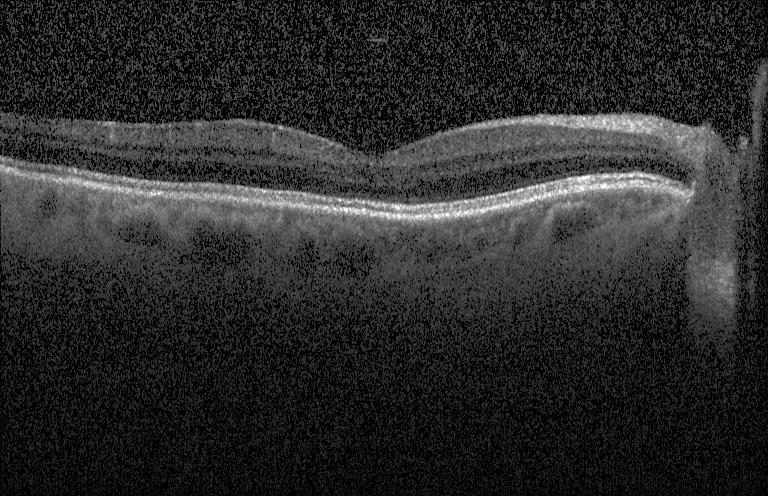

OCT line scan; SD-OCT; through the macula; Heidelberg Spectralis OCT system.
Finding: no CNV, no DME, and no drusen.